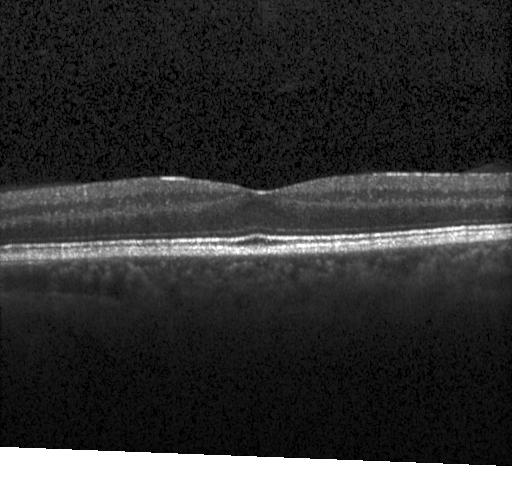

Heidelberg Spectralis OCT system · spectral-domain OCT · optical coherence tomography B-scan · through the macula. Dx: no choroidal neovascularization, no diabetic macular edema, and no drusen.